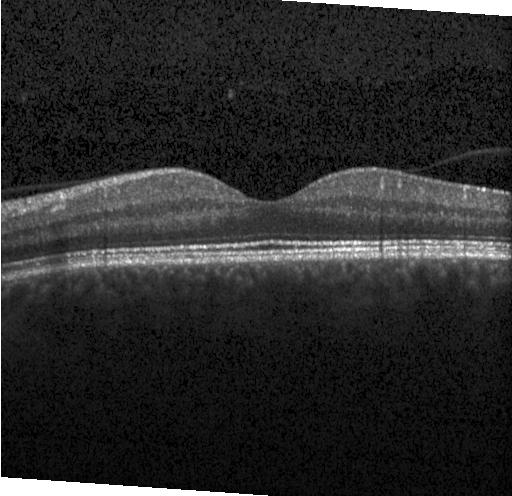
Optical coherence tomography scan.
Finding: no CNV, no DME, and no drusen.